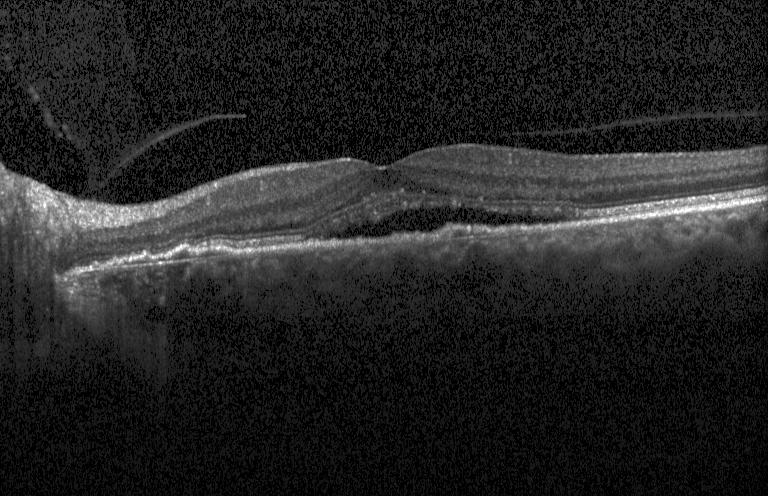
Impression: a choroidal neovascular membrane.